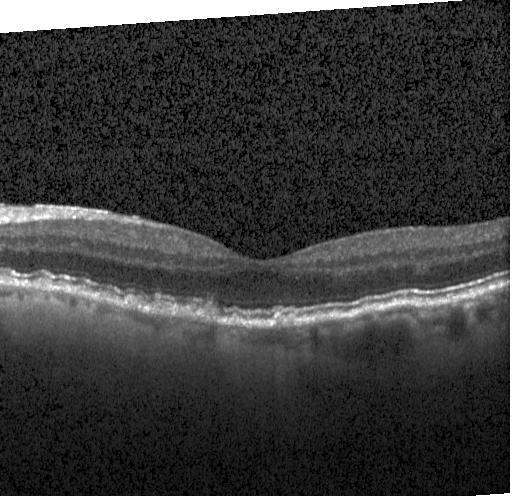

Retinal OCT B-scan; Heidelberg Spectralis OCT system; SD-OCT.
Macular OCT: sub-RPE drusenoid deposits.